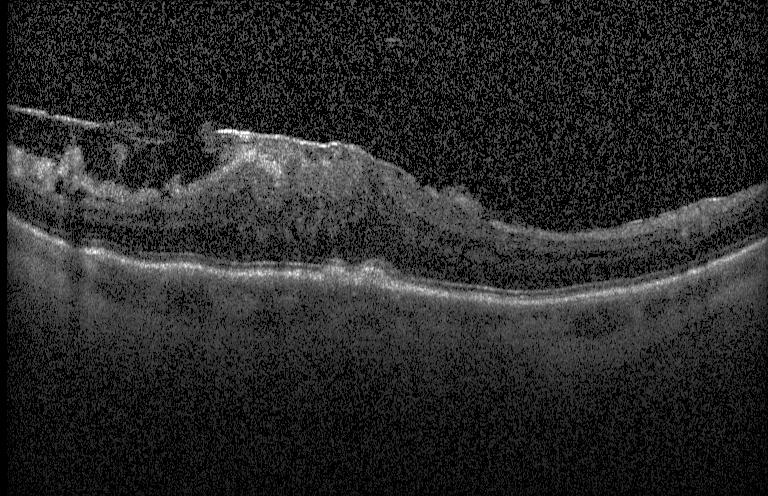

Macular OCT: sub-RPE drusenoid deposits.